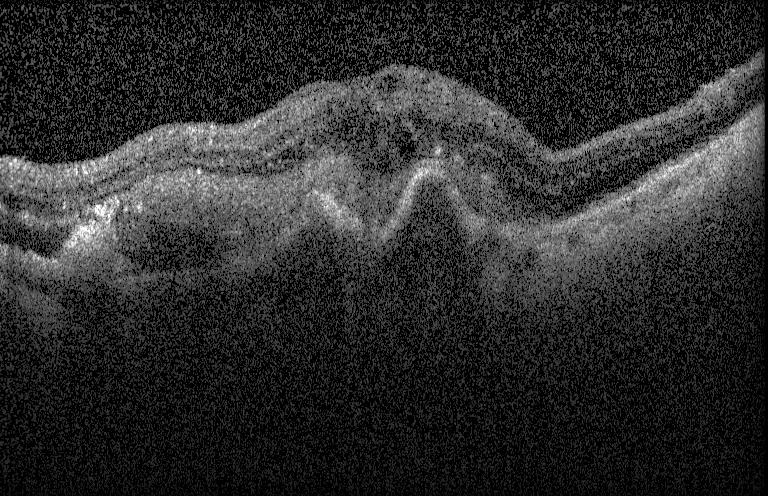

OCT finding: a choroidal neovascular membrane.